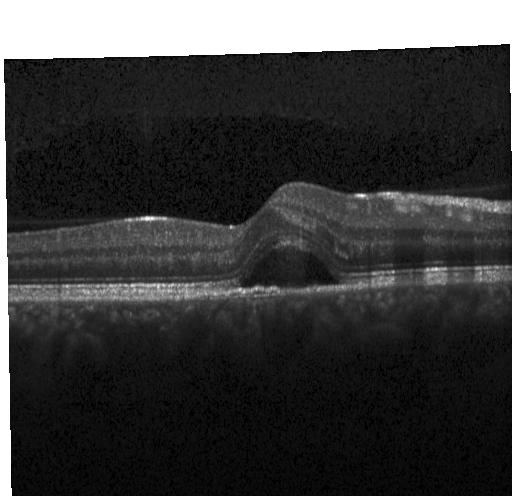 OCT B-scan. Impression: a choroidal neovascular membrane.